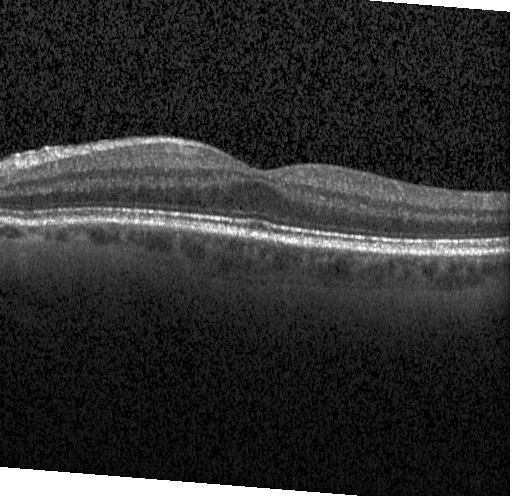

Macular OCT demonstrating no choroidal neovascularization, no diabetic macular edema, and no drusen.